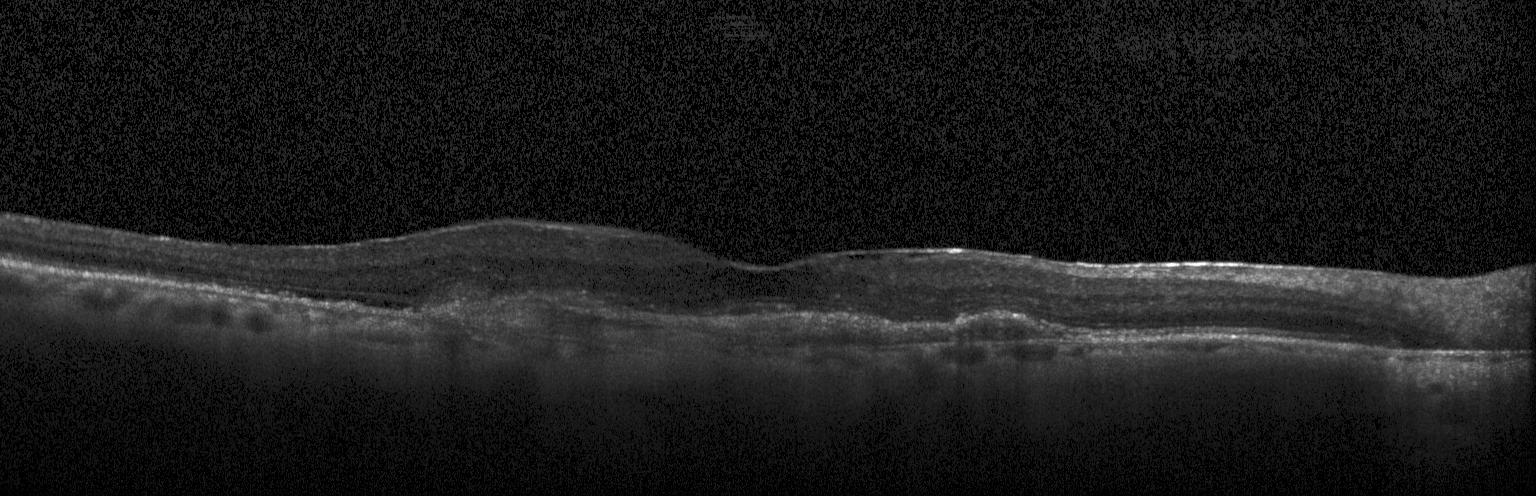

OCT scan showing a choroidal neovascular membrane.